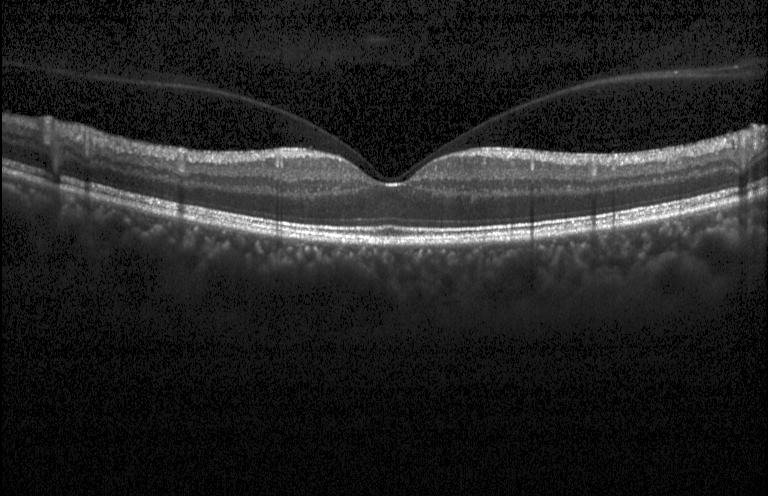 OCT finding: no evidence of CNV, DME, or drusen.